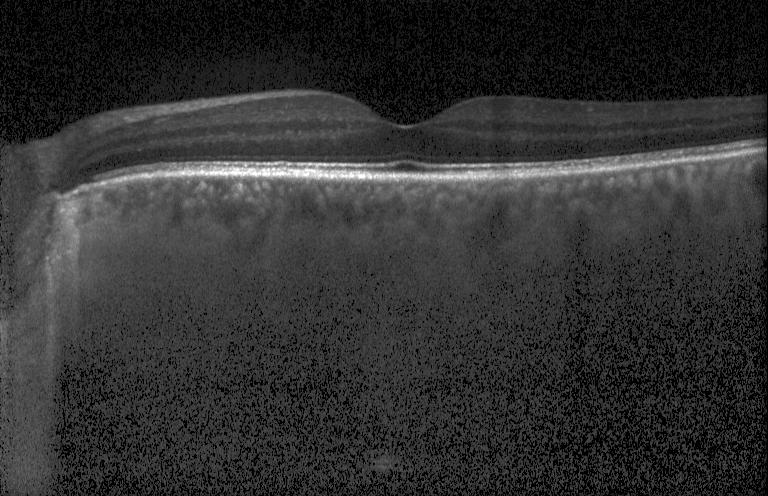
This B-scan demonstrates neither choroidal neovascularization, diabetic macular edema, nor drusen.